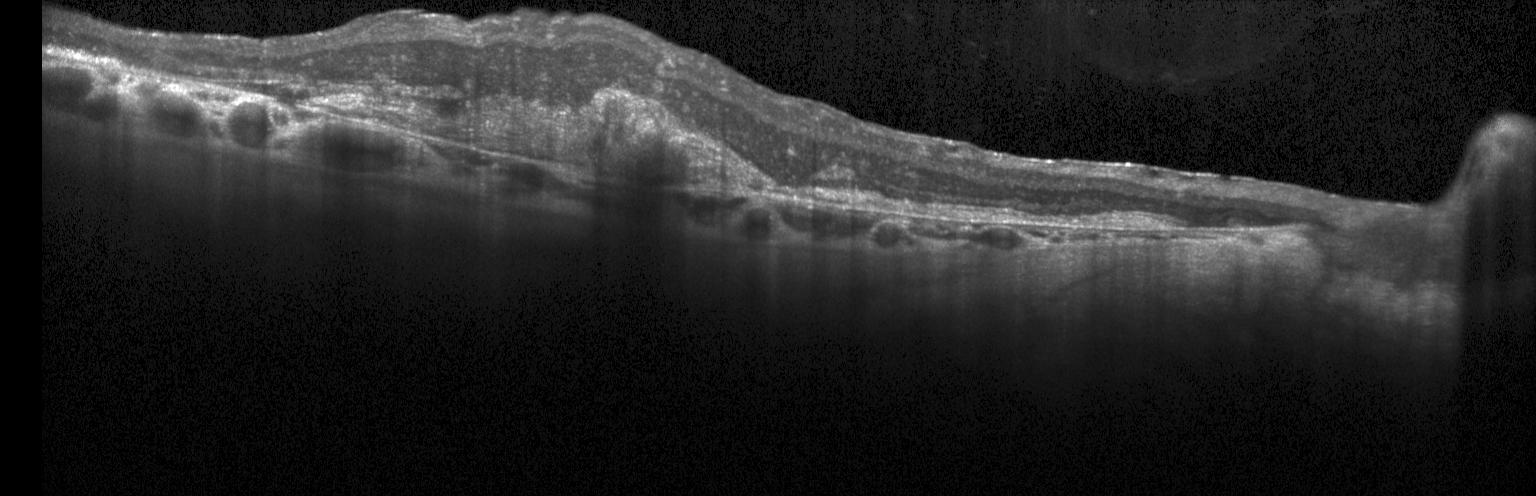 Heidelberg Spectralis OCT system, retinal OCT B-scan. Diagnosis: a choroidal neovascular membrane.